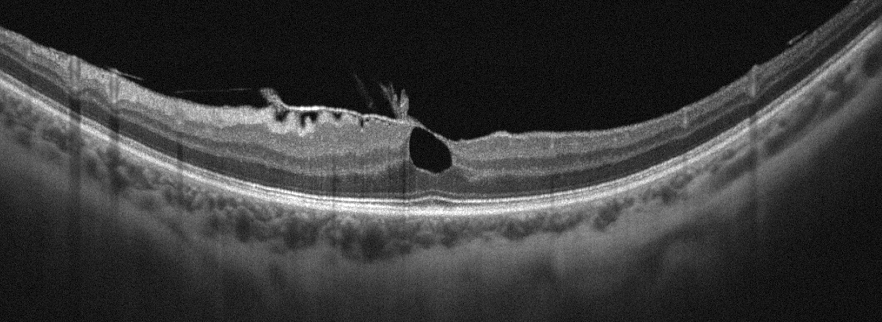
OCT line scan · OS.
Assessment: epiretinal membrane (ERM).